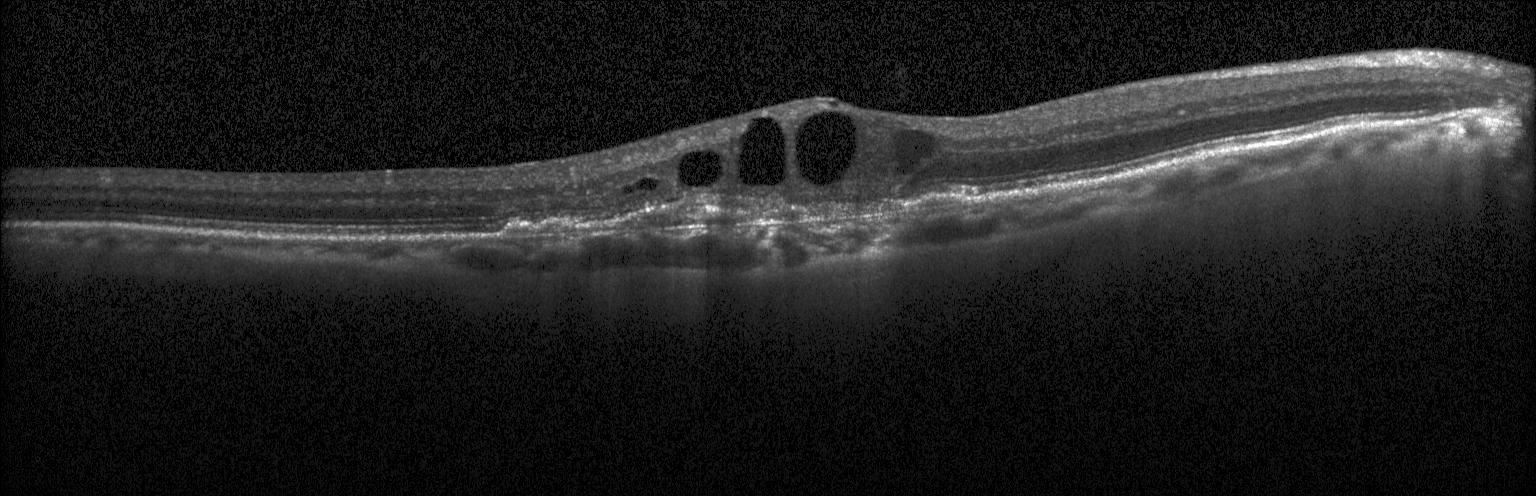

Macular scan. Spectral-domain OCT. Retinal OCT cross-section.
Finding: choroidal neovascularization.